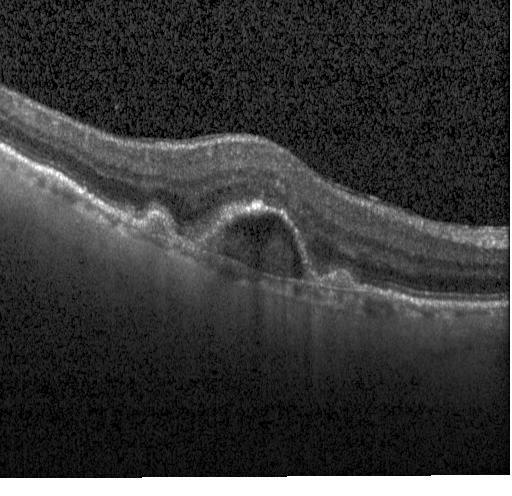 OCT scan showing choroidal neovascularization (CNV).